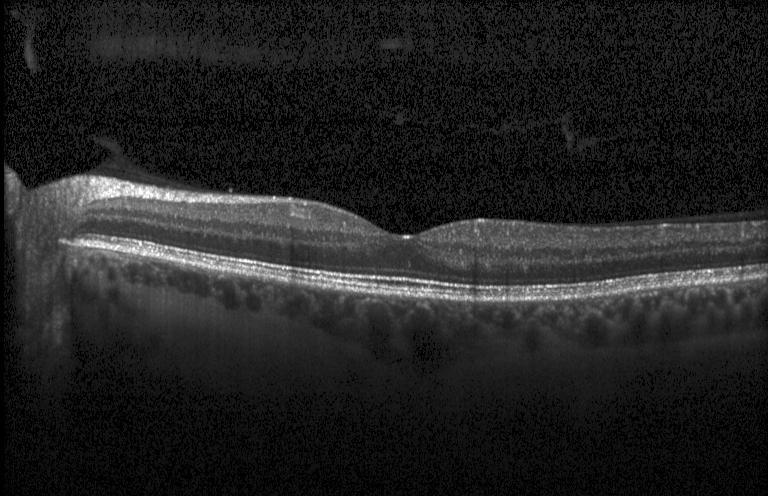
SD-OCT, macular scan, Heidelberg Spectralis, optical coherence tomography scan
No evidence of CNV, DME, or drusen.